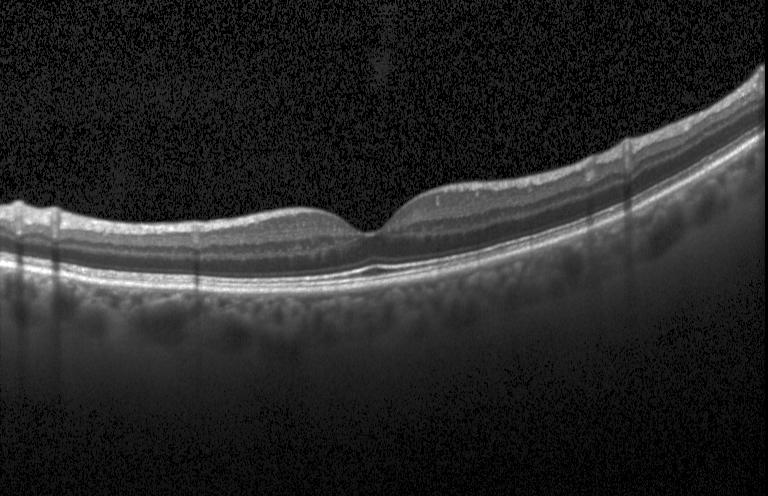
Retinal OCT cross-section · acquired on a Heidelberg Spectralis · macular scan. No choroidal neovascularization, diabetic macular edema, or drusen.